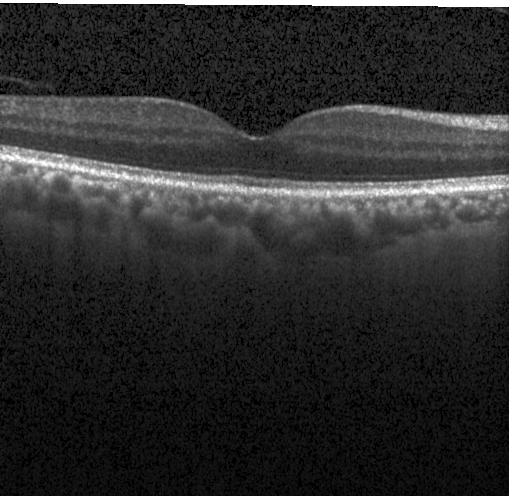 The scan shows neither CNV, DME, nor drusen.